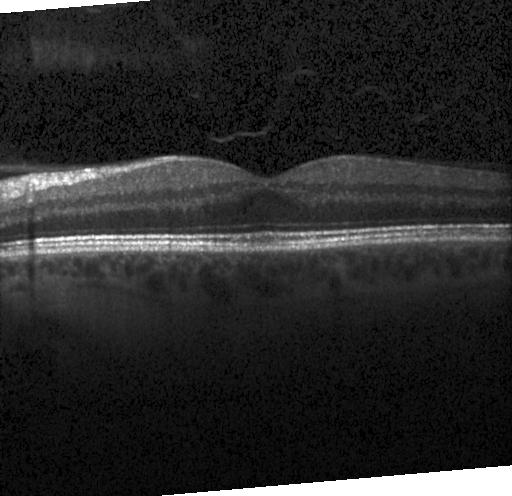 Impression: no choroidal neovascularization, no diabetic macular edema, and no drusen.